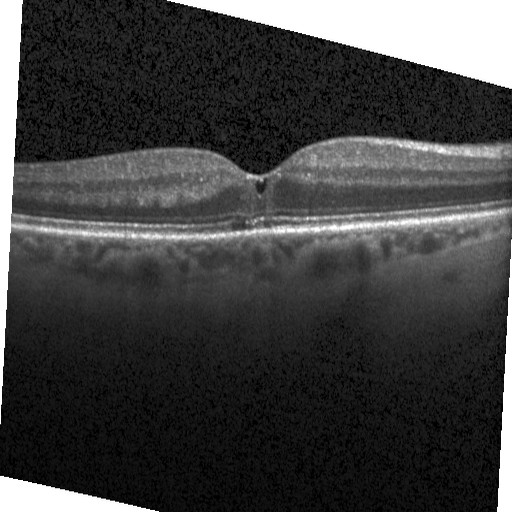
Horizontal scan through the fovea · optical coherence tomography B-scan · instrument: Heidelberg Spectralis
Finding: diabetic macular edema (DME).